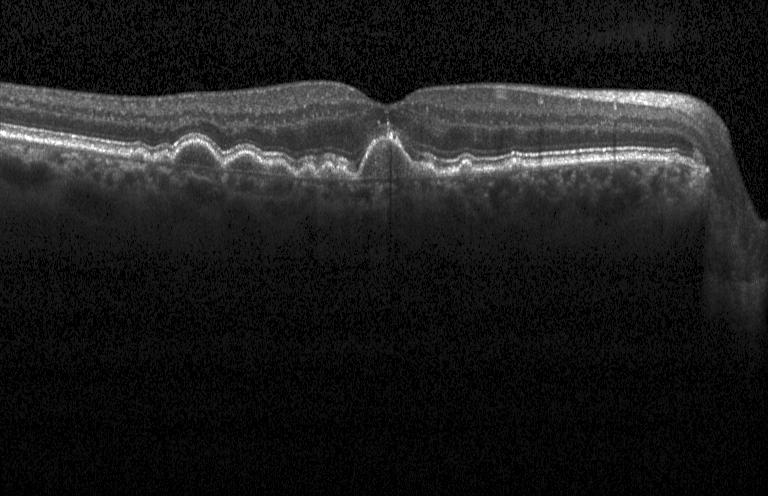

Retinal OCT cross-section showing drusen.